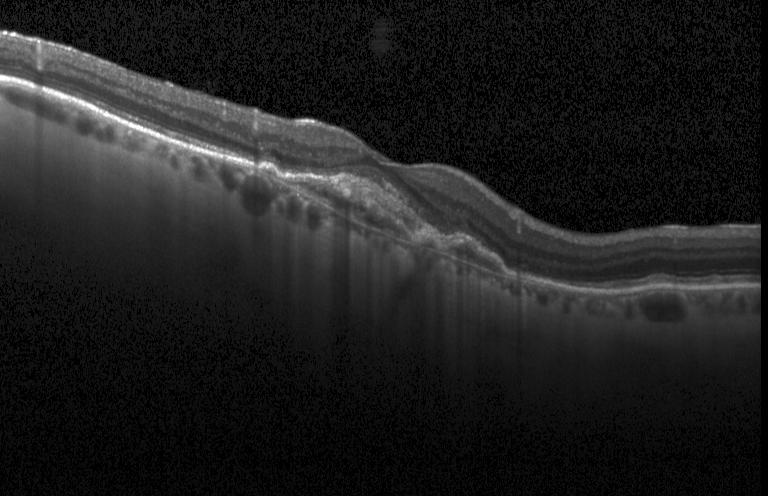

Acquired on a Heidelberg Spectralis. Optical coherence tomography scan. SD-OCT
Finding: a choroidal neovascular membrane.